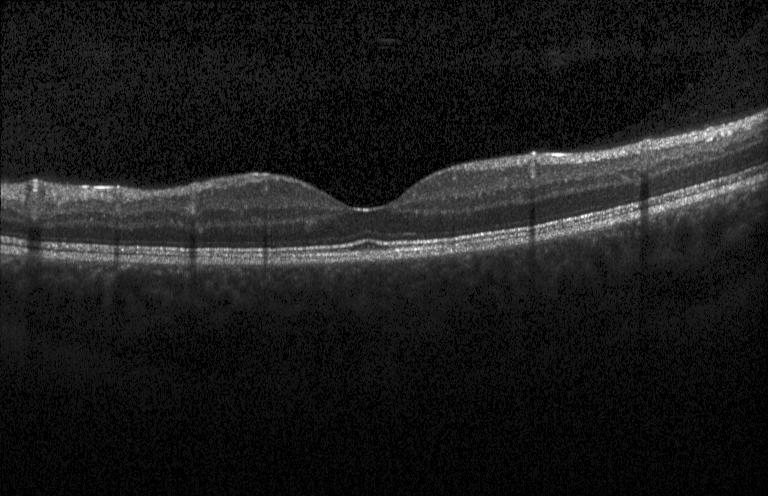 Finding: no choroidal neovascularization, no diabetic macular edema, and no drusen.